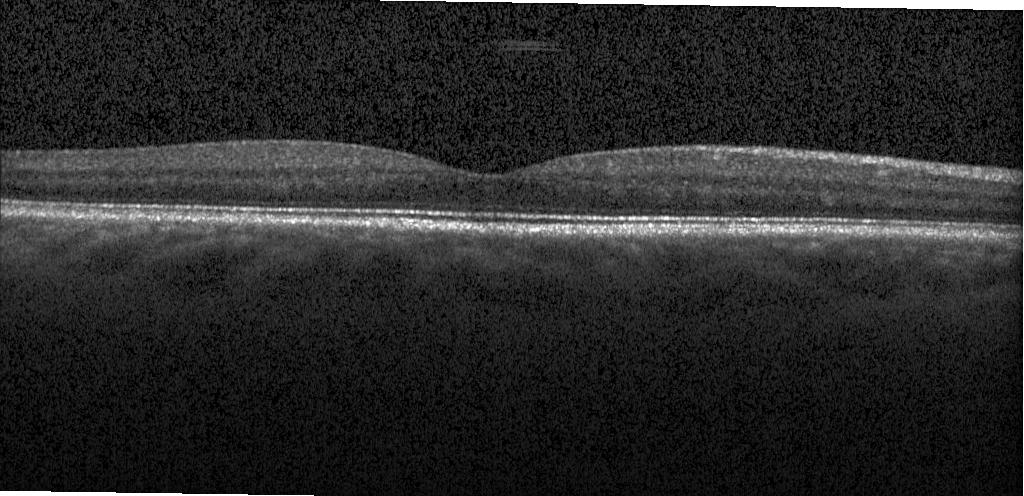

Optical coherence tomography scan.
Assessment: neither CNV, DME, nor drusen.